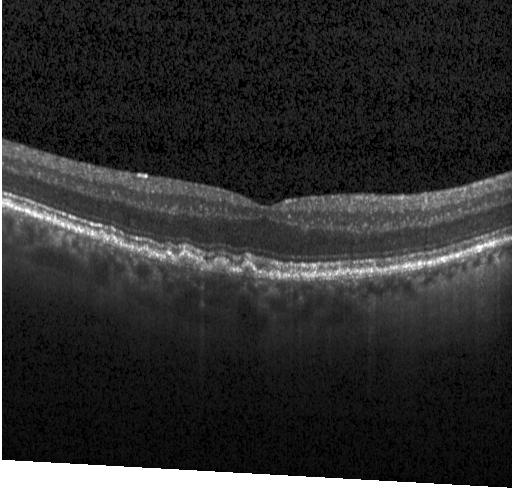
SD-OCT, OCT B-scan, Heidelberg Spectralis
Impression: multiple drusen.